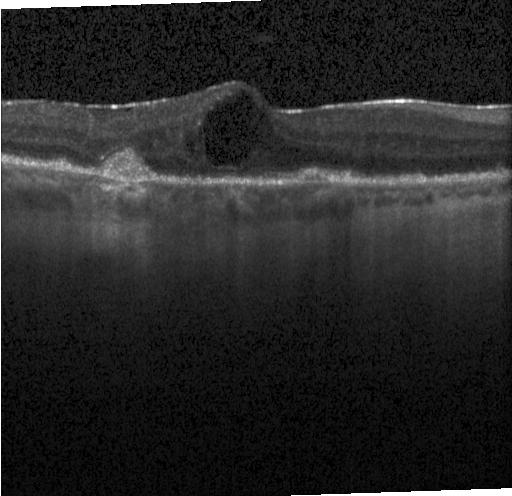 Heidelberg Spectralis OCT system · SD-OCT · OCT B-scan · through the macula. Dx: CNV.